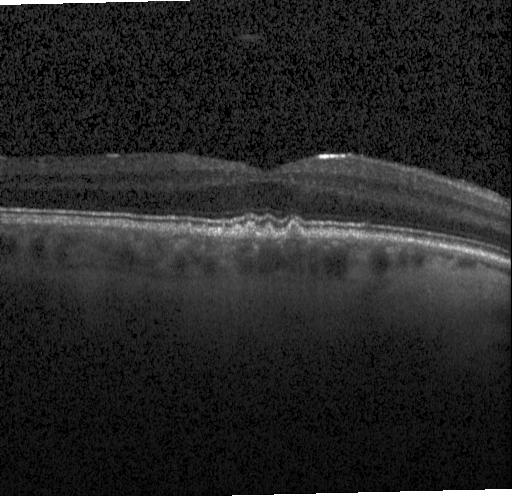 Optical coherence tomography scan; acquired on a Heidelberg Spectralis.
Impression: multiple drusen.